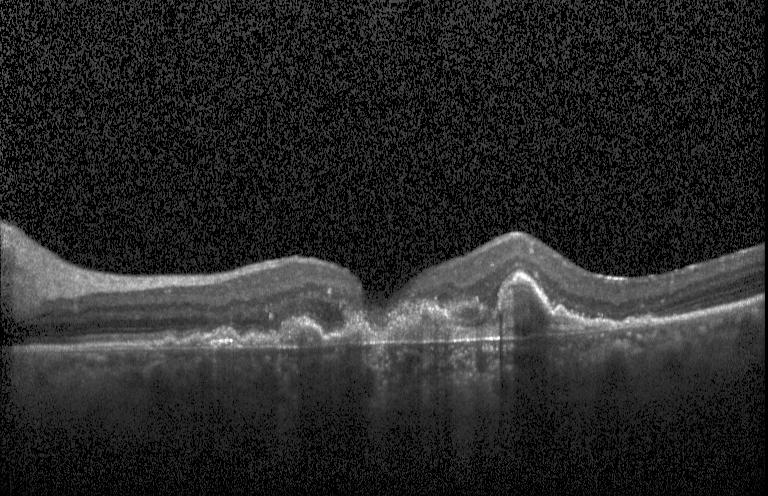

OCT B-scan. Centered on the fovea — Finding: a choroidal neovascular membrane.